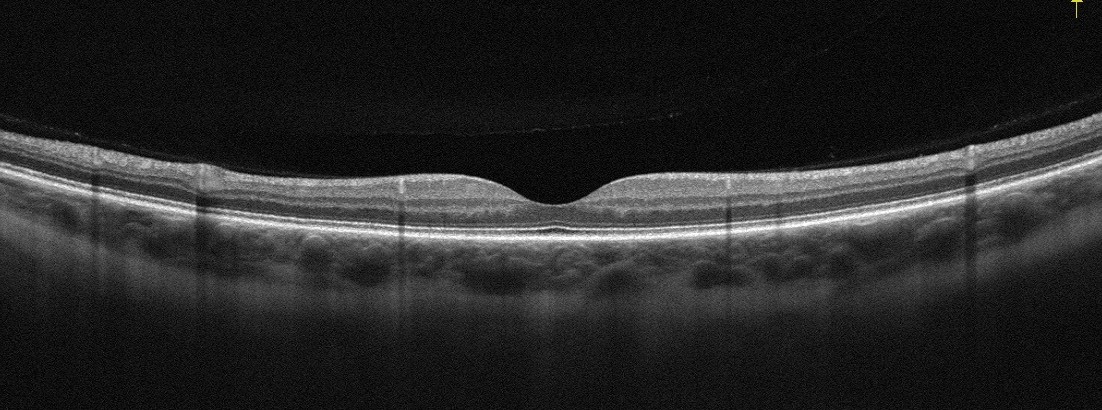 OCT B-scan.
Dx: absence of AMD, DME, ERM, RAO, RVO, and vitreomacular interface disease.